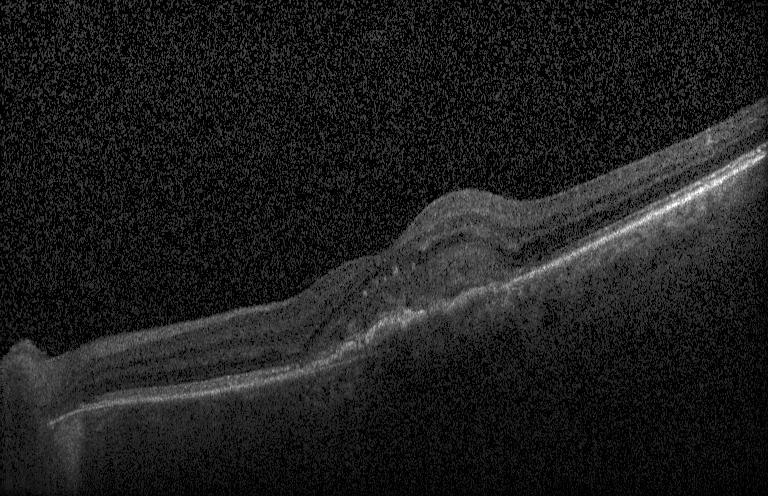 Optical coherence tomography B-scan. Centered on the fovea. SD-OCT.
Assessment: a choroidal neovascular membrane.